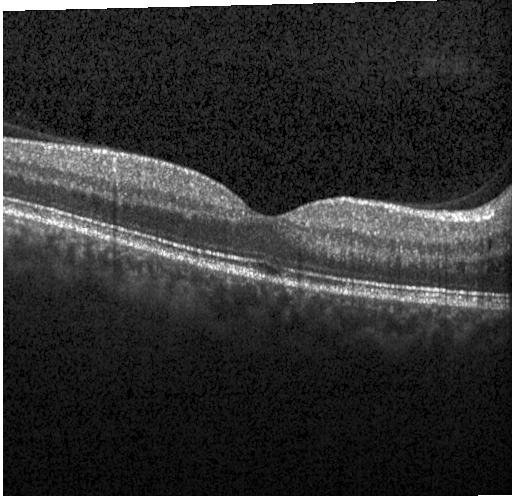

Impression: no choroidal neovascularization, diabetic macular edema, or drusen.